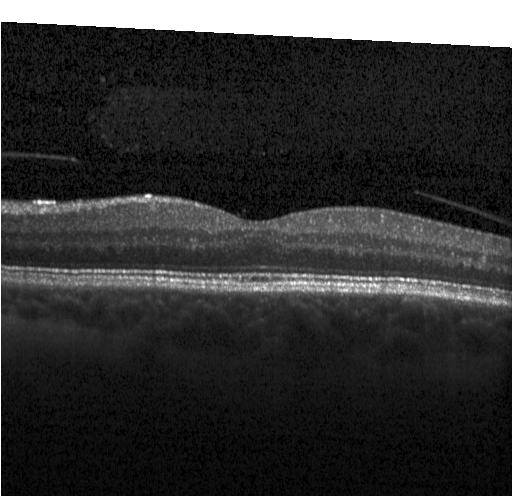 Spectral-domain optical coherence tomography, acquired on a Heidelberg Spectralis, retinal OCT B-scan, fovea-centered
Impression: no CNV, no DME, and no drusen.